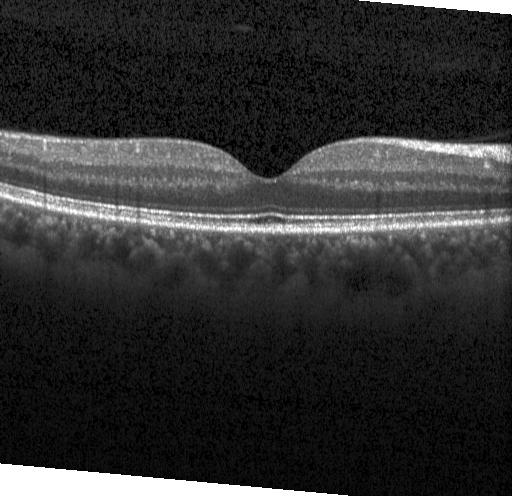

Acquired on a Heidelberg Spectralis · optical coherence tomography B-scan · fovea-centered · spectral-domain OCT — OCT finding: no evidence of choroidal neovascularization, diabetic macular edema, or drusen.